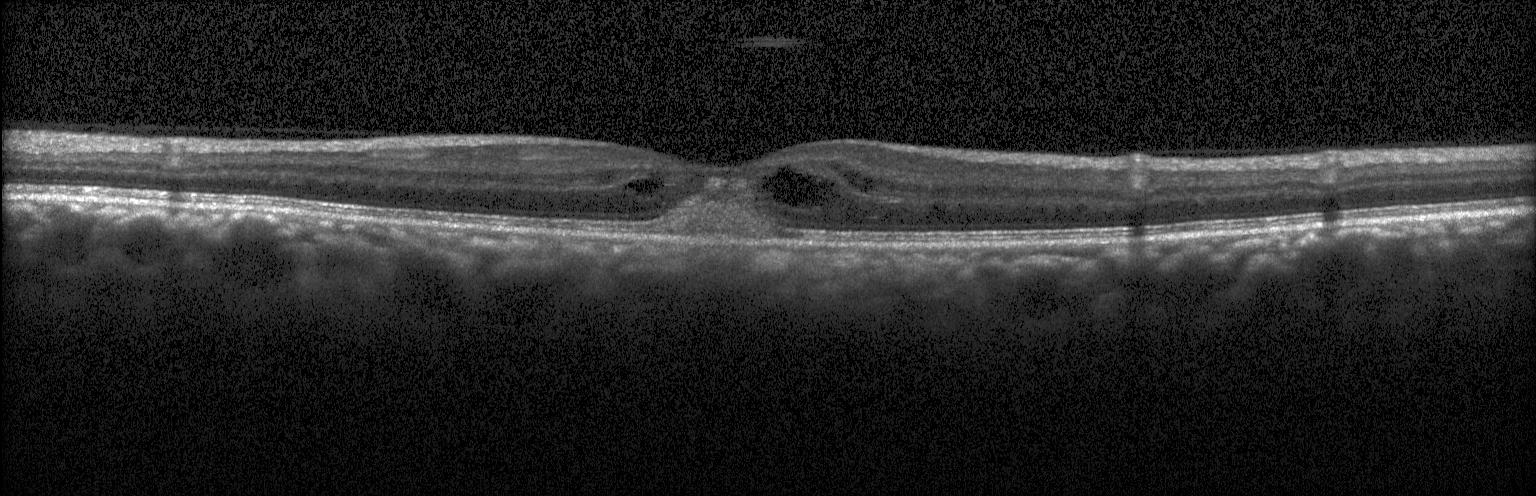 OCT line scan.
Diagnosis: a choroidal neovascular membrane.